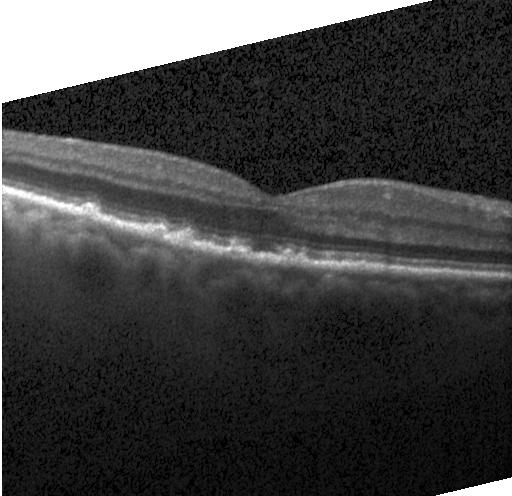 OCT B-scan; Heidelberg Spectralis; centered on the fovea — This B-scan demonstrates drusen.